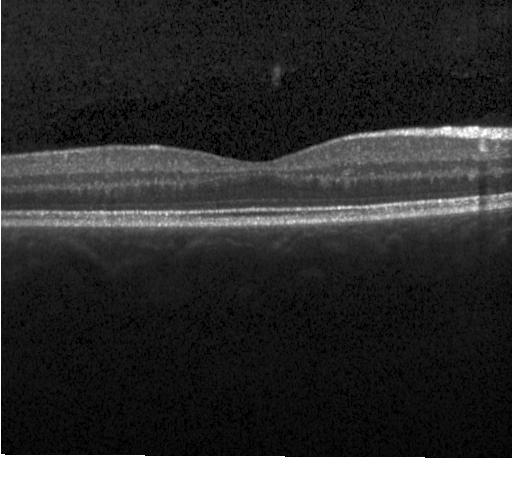
Finding: no CNV, no DME, and no drusen.